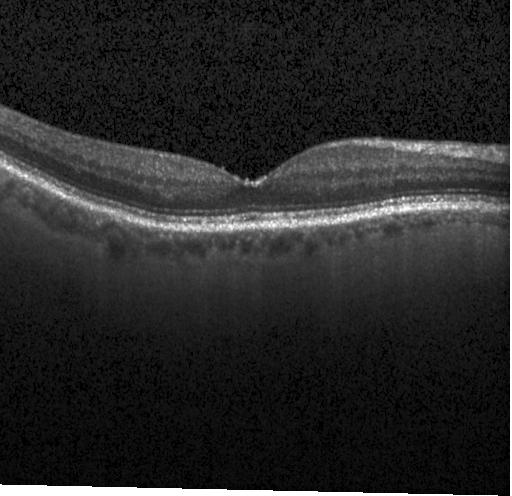

Finding: neither CNV, DME, nor drusen.